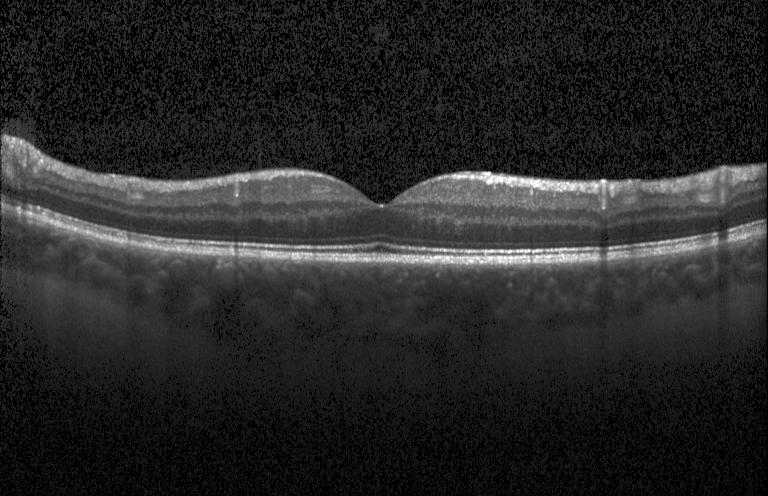

The scan shows no choroidal neovascularization, no diabetic macular edema, and no drusen.